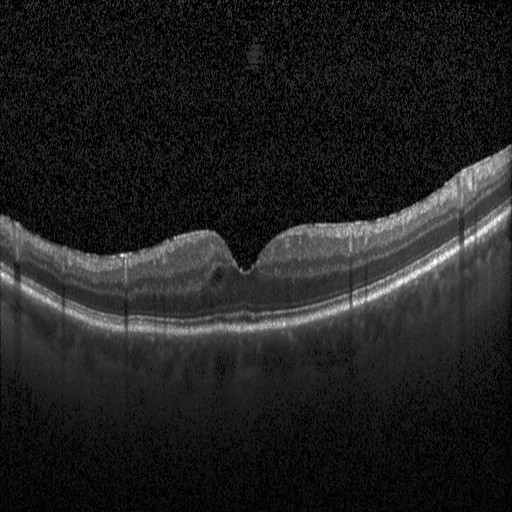 Retinal OCT cross-section; macular scan; spectral-domain optical coherence tomography. Impression: diabetic macular edema.